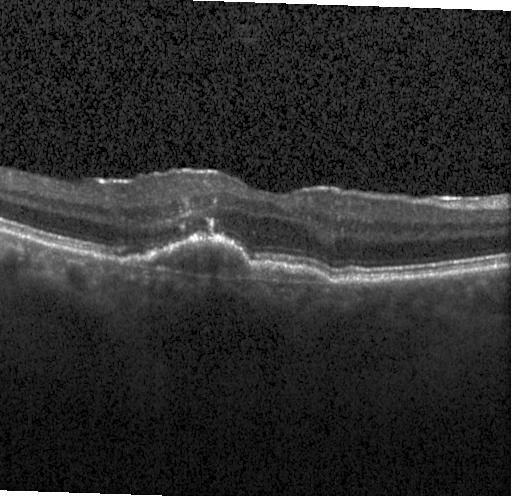
Dx: a choroidal neovascular membrane.